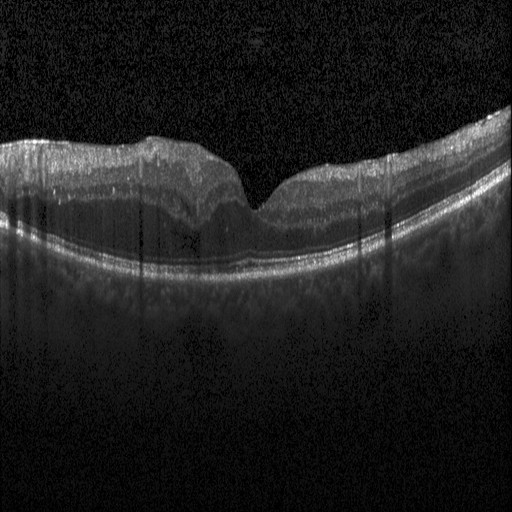
Spectral-domain optical coherence tomography, retinal OCT cross-section, Heidelberg Spectralis OCT system
Finding: diabetic macular edema.